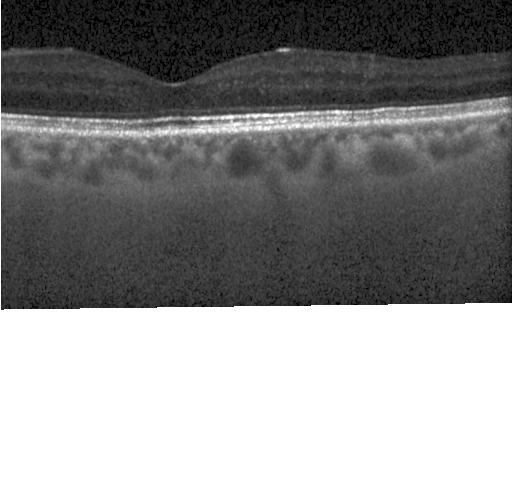
Macular scan; OCT B-scan
The scan shows no evidence of choroidal neovascularization, diabetic macular edema, or drusen.